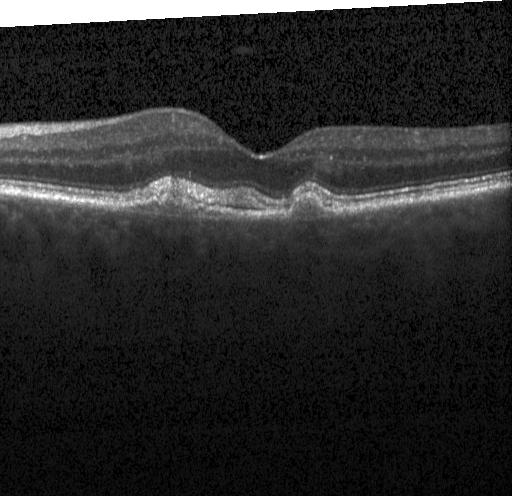

Optical coherence tomography B-scan. Instrument: Heidelberg Spectralis. Spectral-domain optical coherence tomography.
Diagnosis: choroidal neovascularization (CNV).